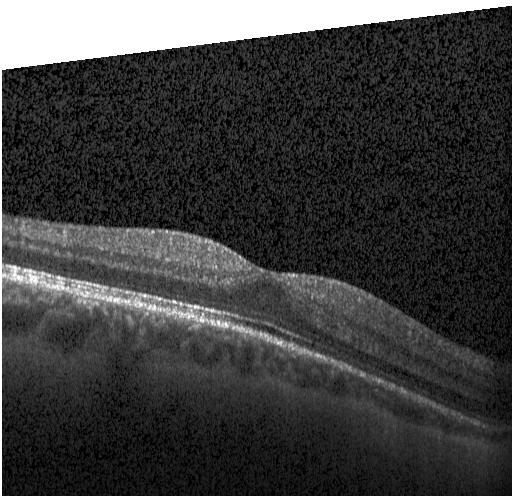
Finding: neither choroidal neovascularization, diabetic macular edema, nor drusen.